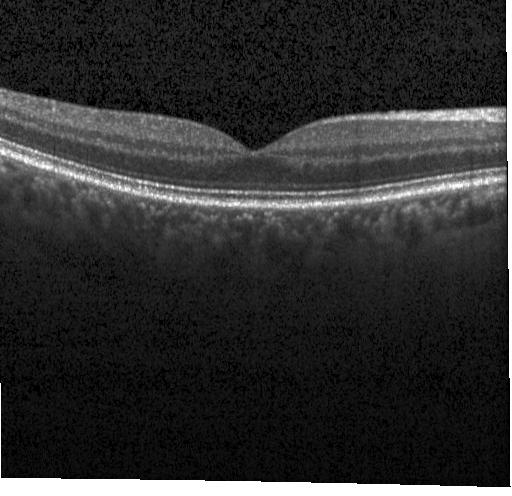

This B-scan demonstrates no CNV, DME, or drusen.